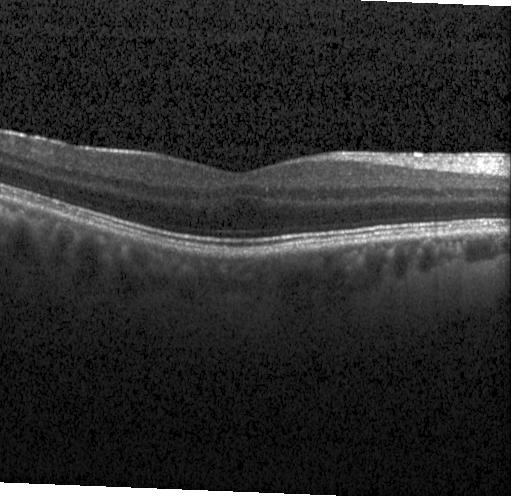 Finding: no evidence of choroidal neovascularization, diabetic macular edema, or drusen.